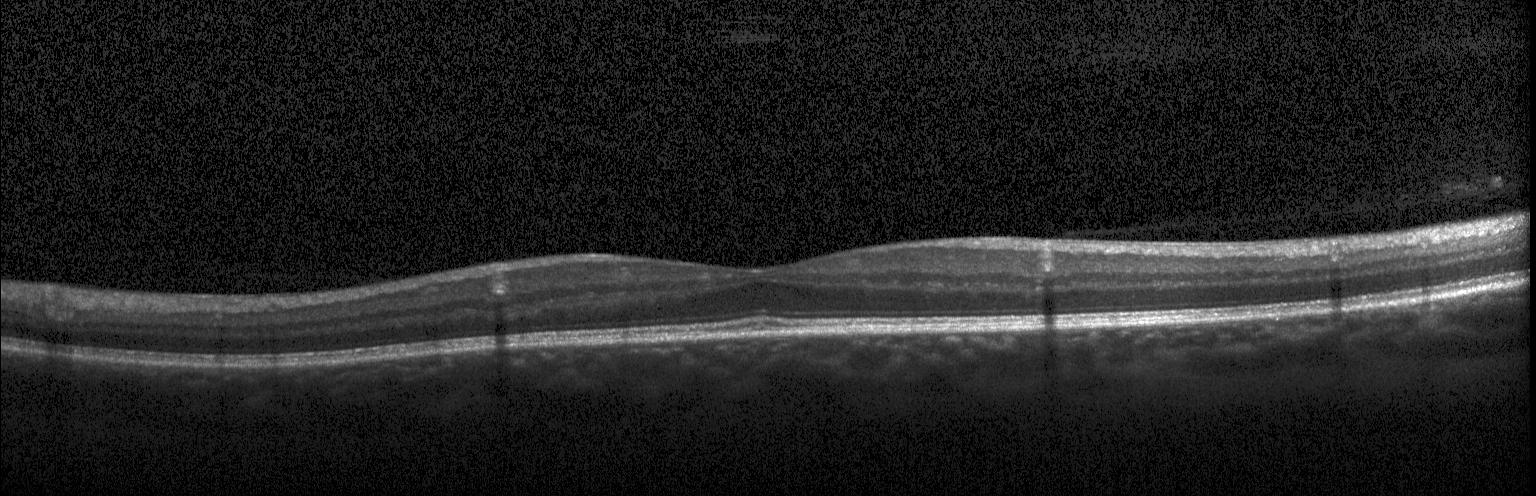

OCT line scan; centered on the fovea; acquired on a Heidelberg Spectralis; SD-OCT.
Finding: no choroidal neovascularization, no diabetic macular edema, and no drusen.